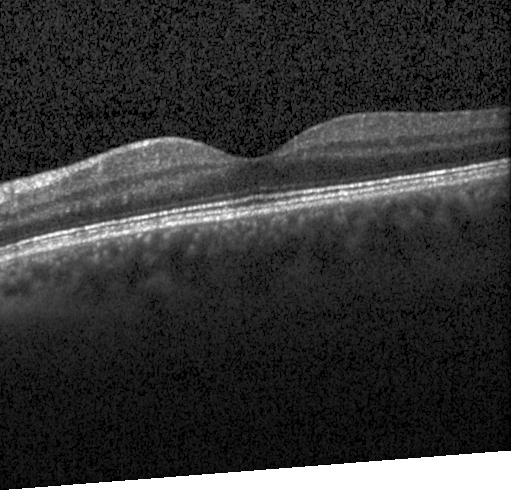
Fovea-centered; optical coherence tomography B-scan; Heidelberg Spectralis OCT system
This B-scan demonstrates no CNV, DME, or drusen.